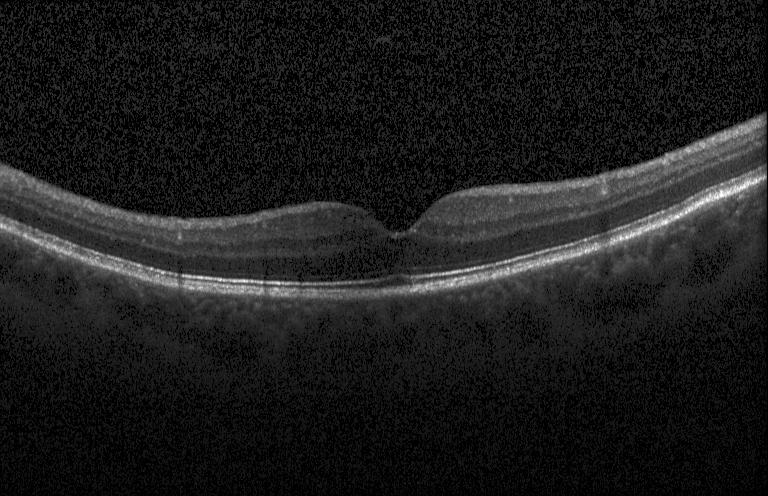

OCT line scan. Macular scan — Finding: no CNV, no DME, and no drusen.